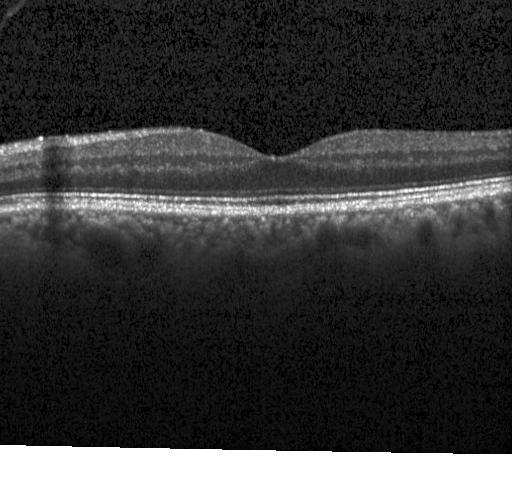 Heidelberg Spectralis, SD-OCT, OCT line scan
Diagnosis: no evidence of choroidal neovascularization, diabetic macular edema, or drusen.